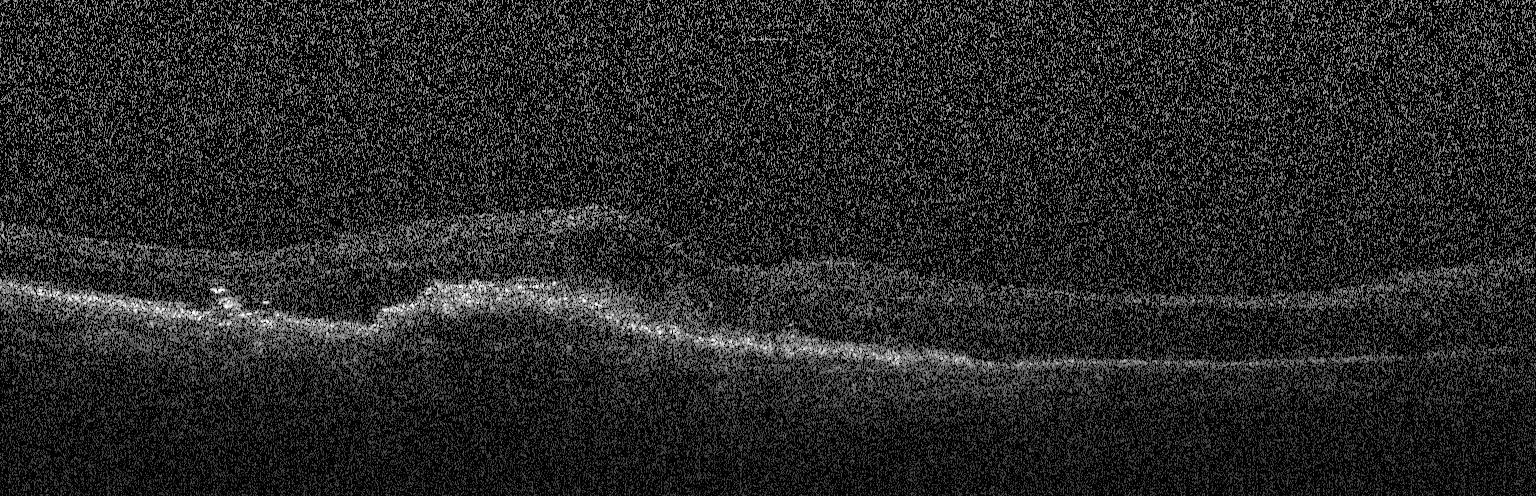
This B-scan demonstrates a choroidal neovascular membrane.